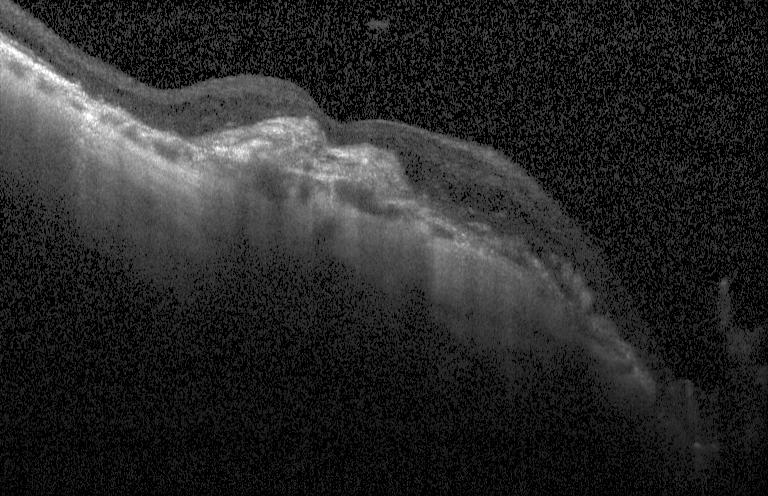 SD-OCT. OCT line scan — Finding: choroidal neovascularization.